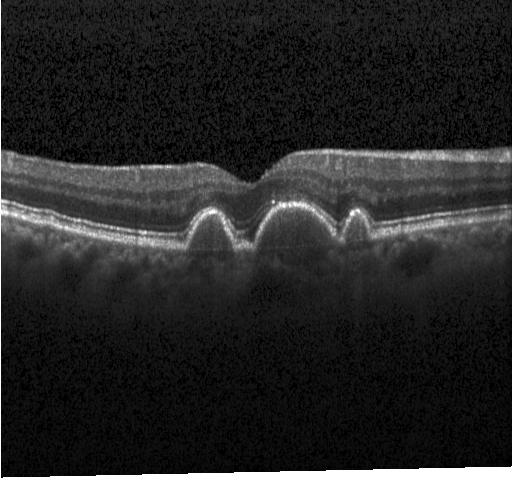 Dx: multiple drusen.